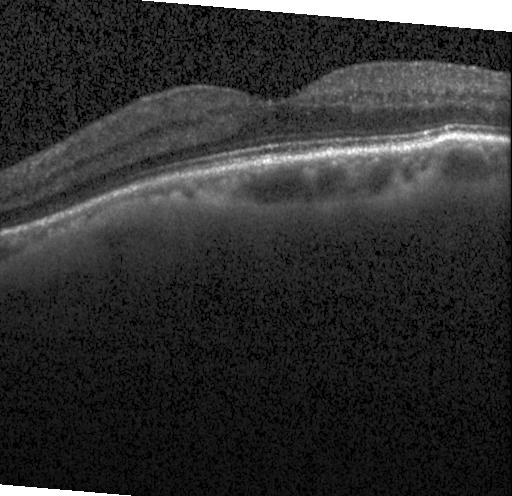 Macular OCT: no choroidal neovascularization, no diabetic macular edema, and no drusen.